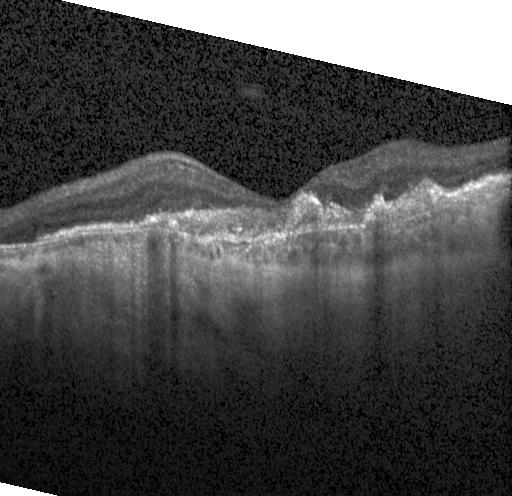
Acquired on a Heidelberg Spectralis · OCT B-scan · centered on the fovea.
OCT finding: CNV.